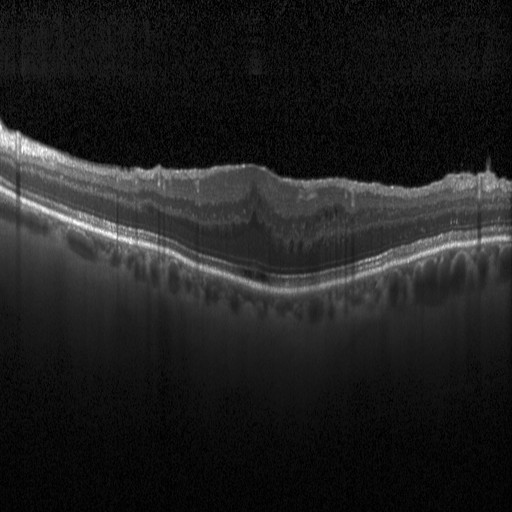 Diagnosis: diabetic macular edema.